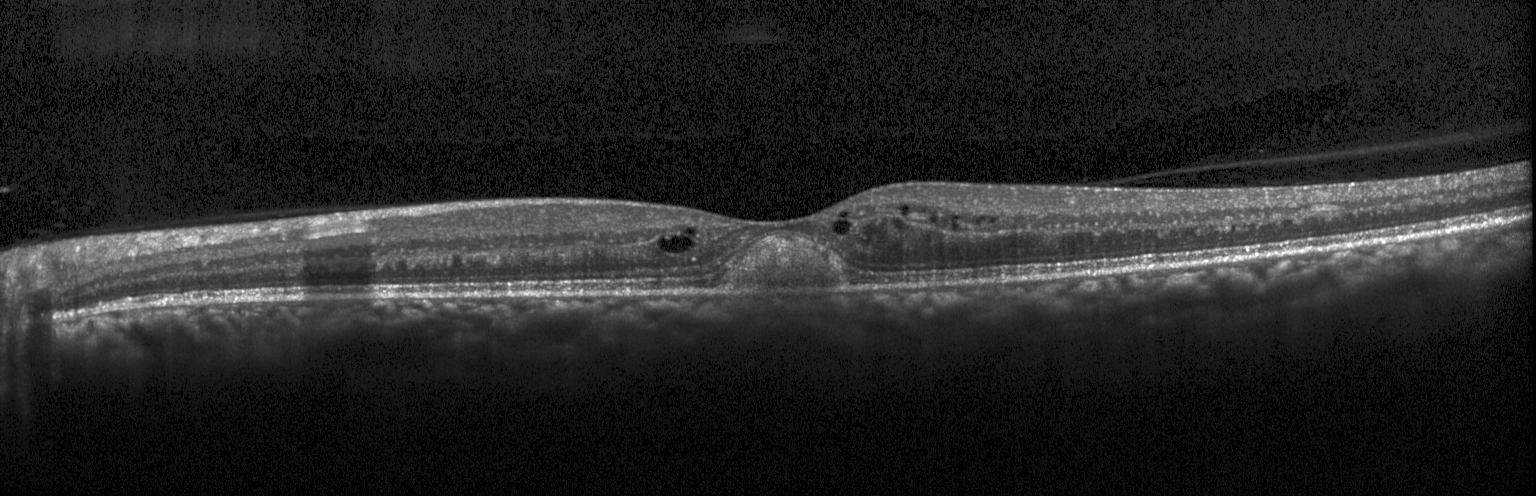 Retinal OCT B-scan
Impression: a choroidal neovascular membrane.